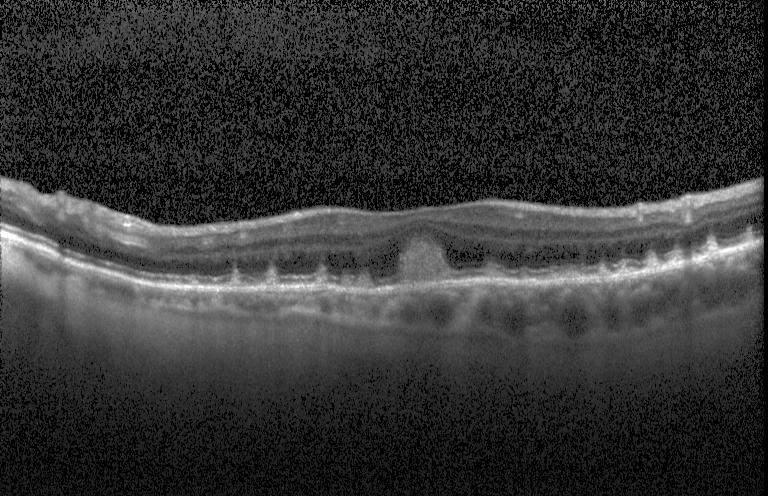 Impression: a choroidal neovascular membrane.